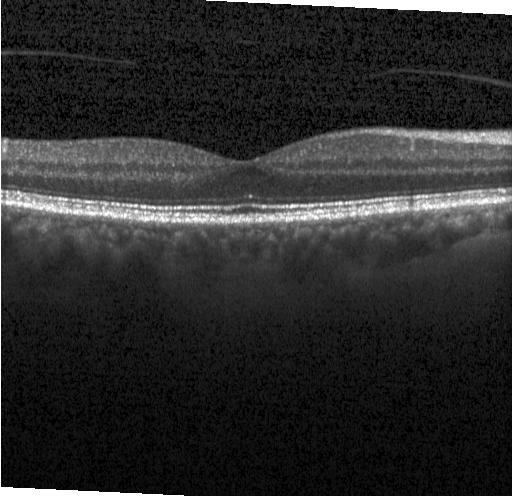 Acquired on a Heidelberg Spectralis, OCT line scan, centered on the fovea — Diagnosis: no choroidal neovascularization, no diabetic macular edema, and no drusen.